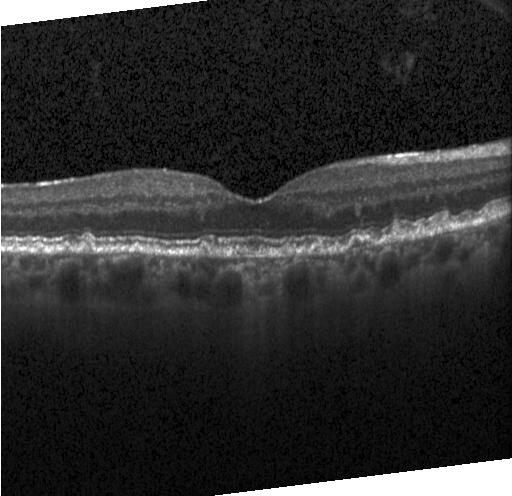
Multiple drusen.